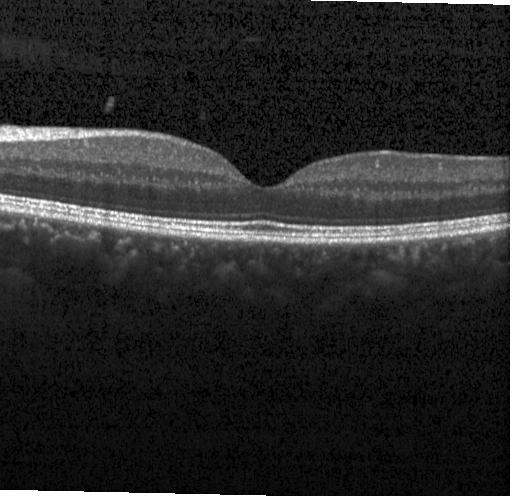
OCT finding: no evidence of choroidal neovascularization, diabetic macular edema, or drusen.